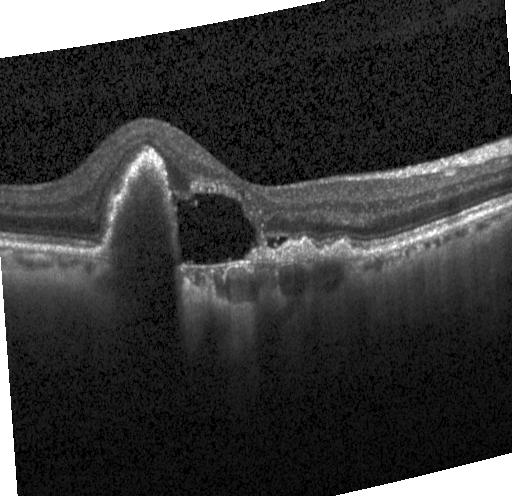
Optical coherence tomography B-scan · Heidelberg Spectralis. Diagnosis: a choroidal neovascular membrane.